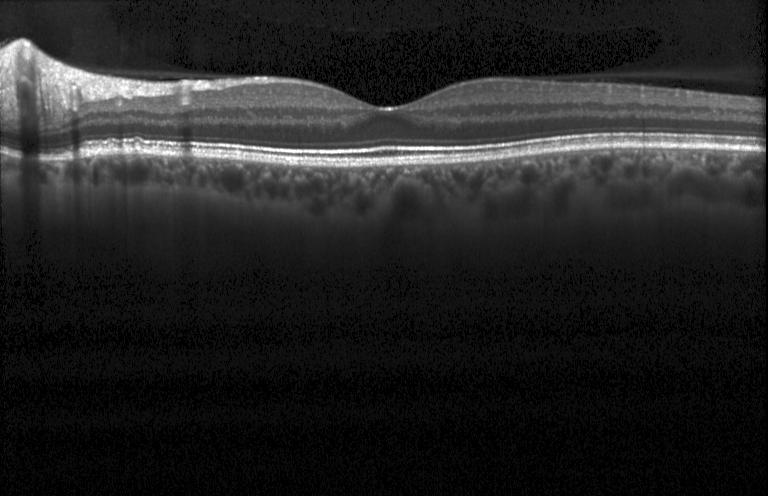
Spectral-domain OCT, macular scan, OCT B-scan, Heidelberg Spectralis.
Multiple drusen.